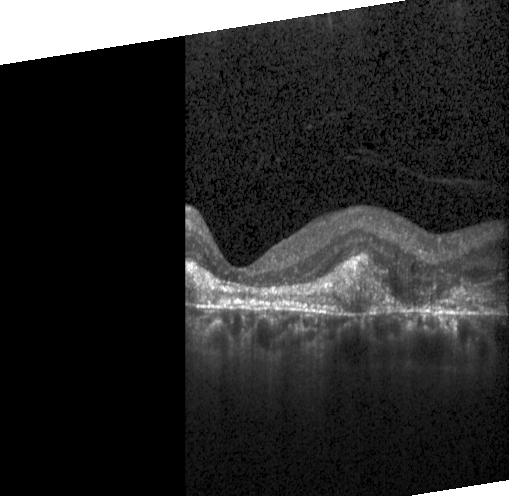

Optical coherence tomography scan.
OCT finding: CNV.